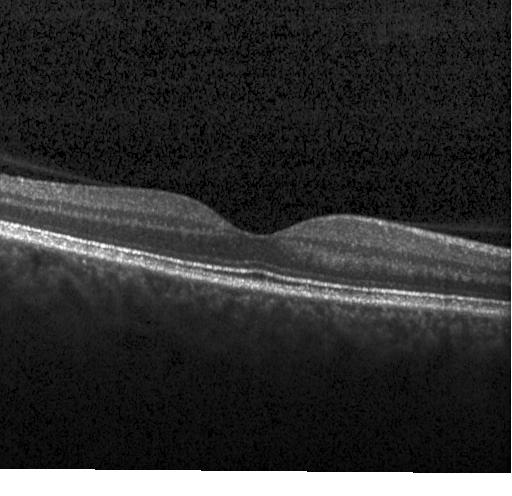

Macular OCT demonstrating no evidence of CNV, DME, or drusen.